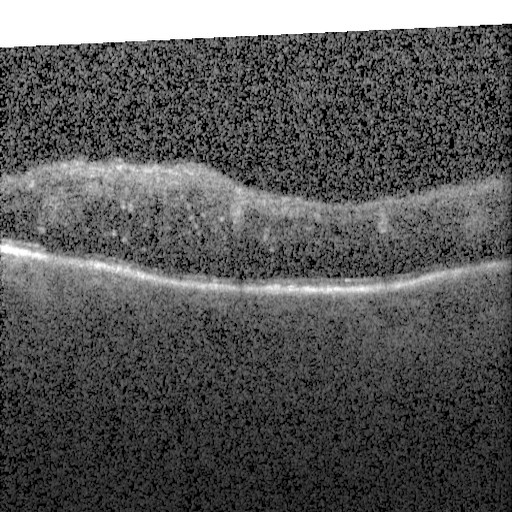 Spectral-domain OCT · optical coherence tomography B-scan.
Finding: diabetic macular edema.